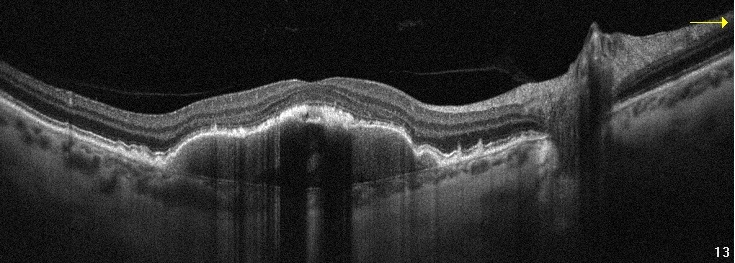 Retinal OCT cross-section; instrument: Optovue Avanti RTVue XR; macular scan.
OCT finding: age-related macular degeneration (AMD).